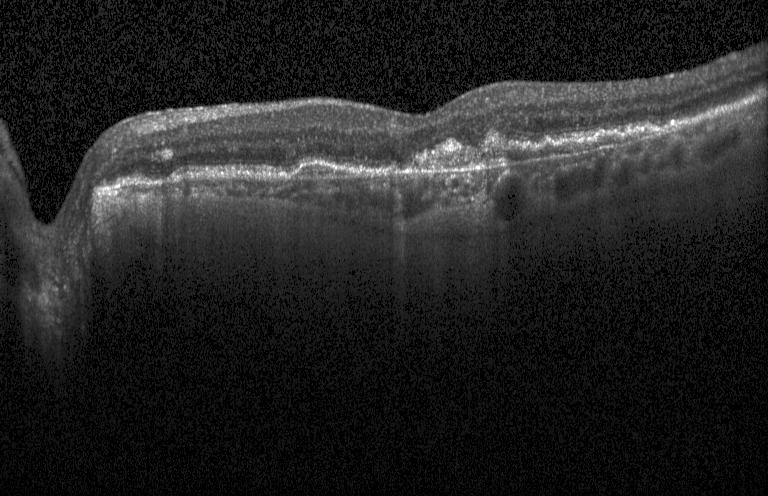
Diagnosis: a choroidal neovascular membrane.